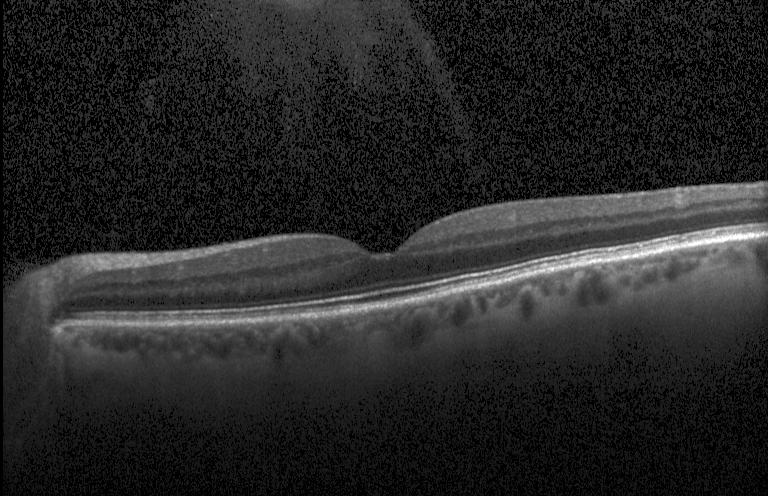
Impression: no CNV, no DME, and no drusen.